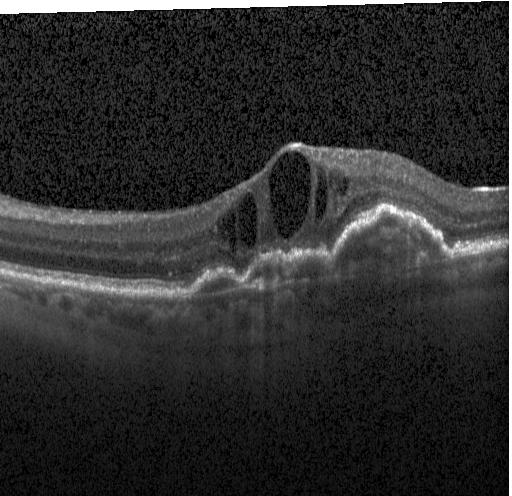 OCT finding: CNV.